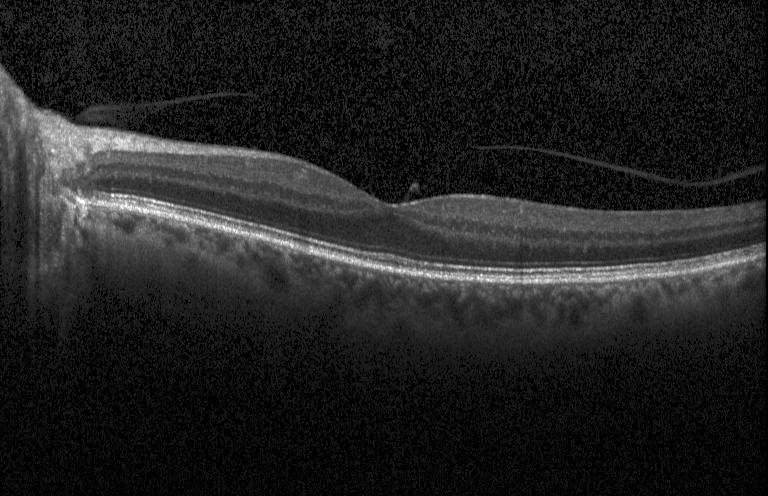
OCT line scan, instrument: Heidelberg Spectralis — OCT finding: neither choroidal neovascularization, diabetic macular edema, nor drusen.